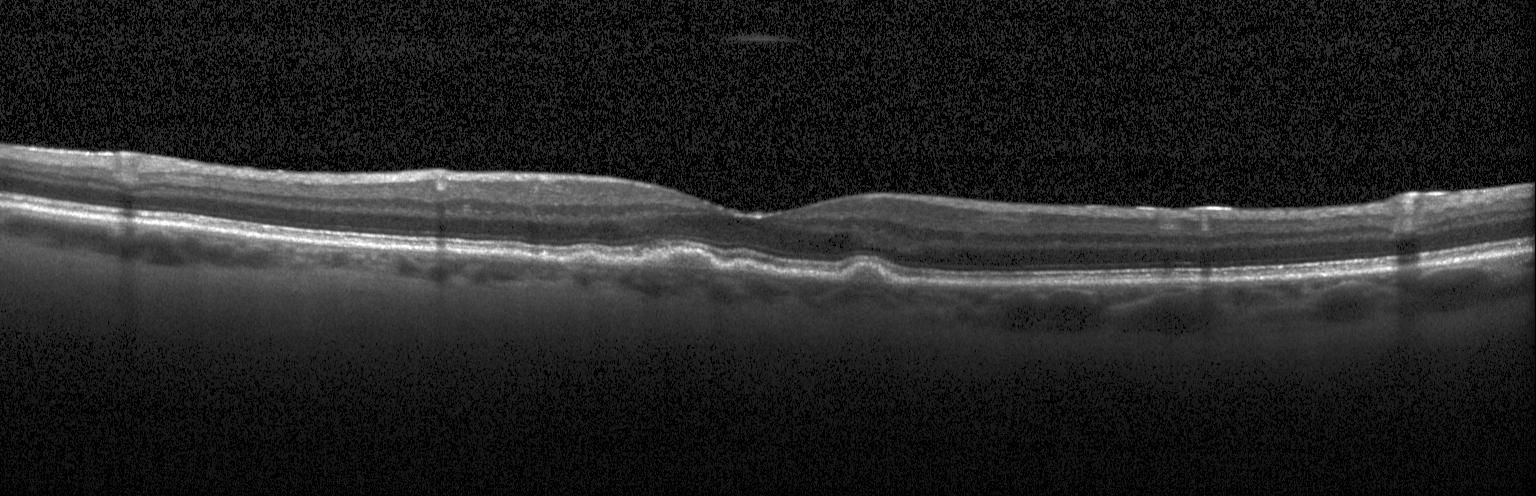 Macular OCT: multiple drusen.